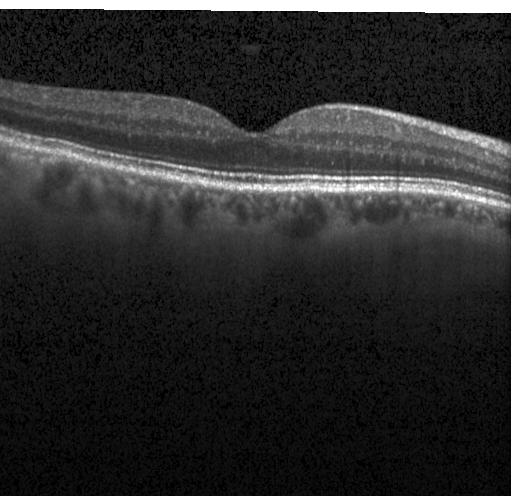
Optical coherence tomography B-scan. Heidelberg Spectralis. Spectral-domain OCT. Horizontal scan through the fovea
OCT finding: no evidence of CNV, DME, or drusen.